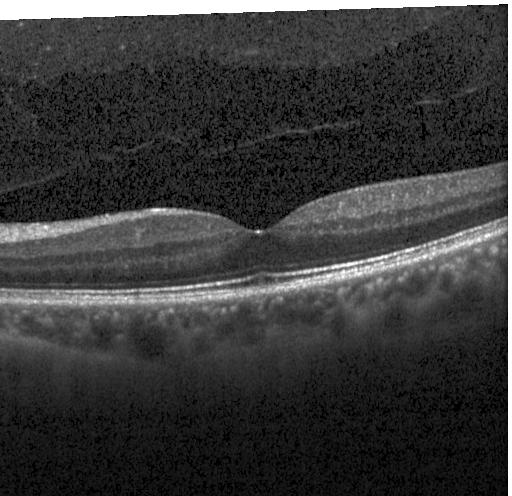 Retinal OCT cross-section · through the macula. OCT finding: no CNV, DME, or drusen.